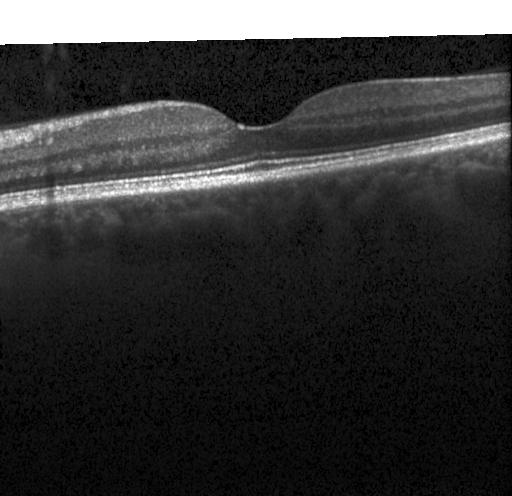

Retinal OCT B-scan. SD-OCT. Horizontal scan through the fovea.
Macular OCT: neither choroidal neovascularization, diabetic macular edema, nor drusen.